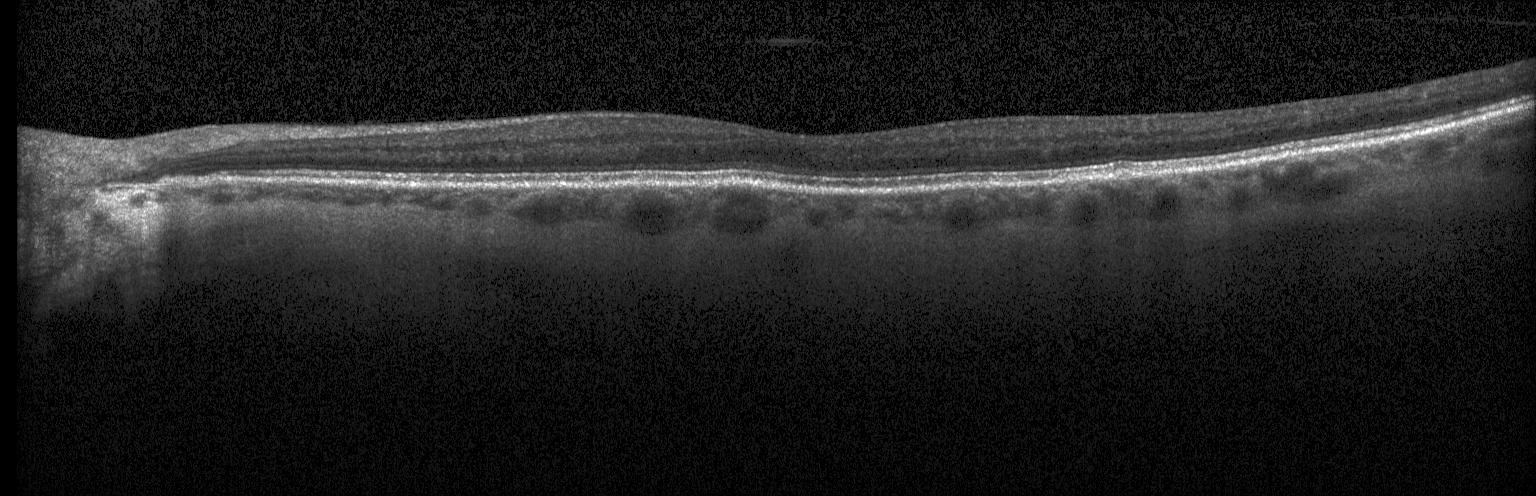

No evidence of CNV, DME, or drusen.